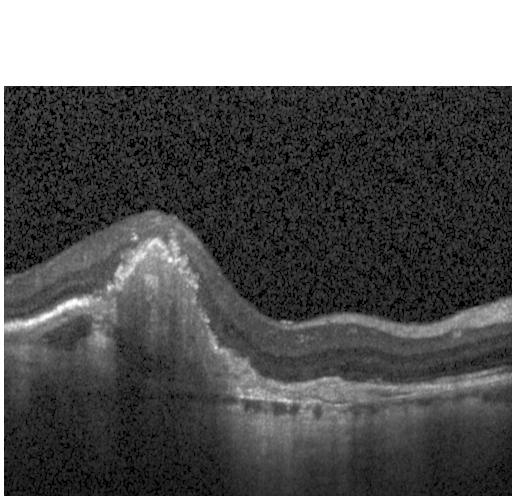

Optical coherence tomography scan; horizontal scan through the fovea
Finding: a choroidal neovascular membrane.